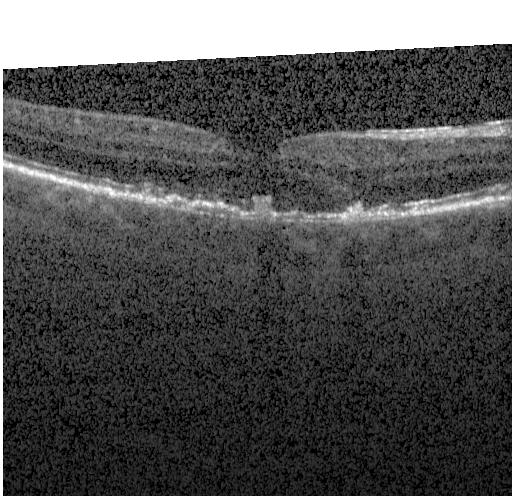 OCT B-scan showing choroidal neovascularization.